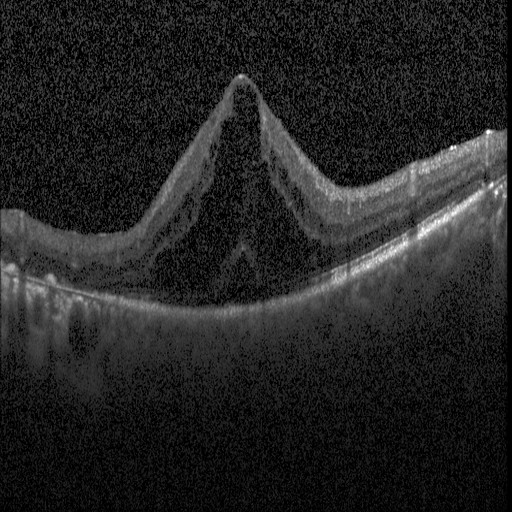
Dx: diabetic macular edema.